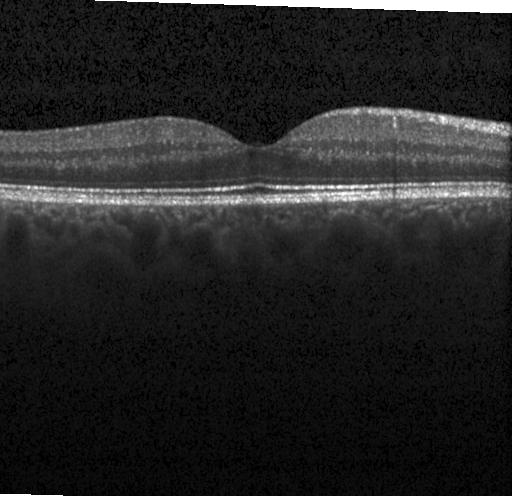
This B-scan demonstrates no evidence of choroidal neovascularization, diabetic macular edema, or drusen.